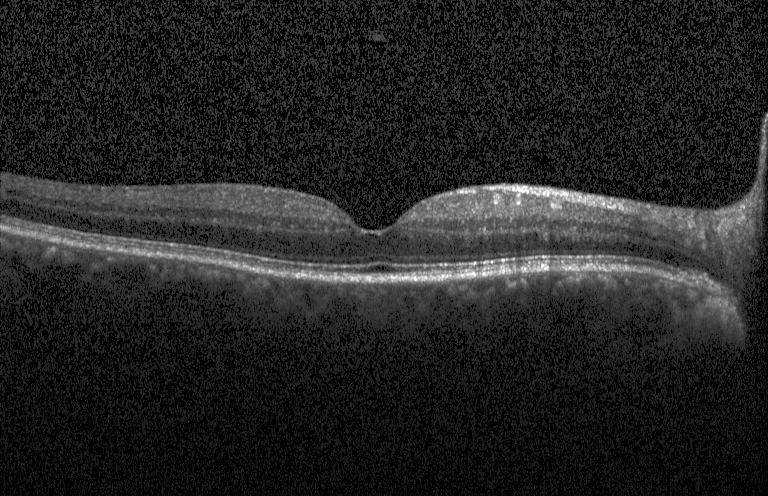 Optical coherence tomography scan
No evidence of CNV, DME, or drusen.